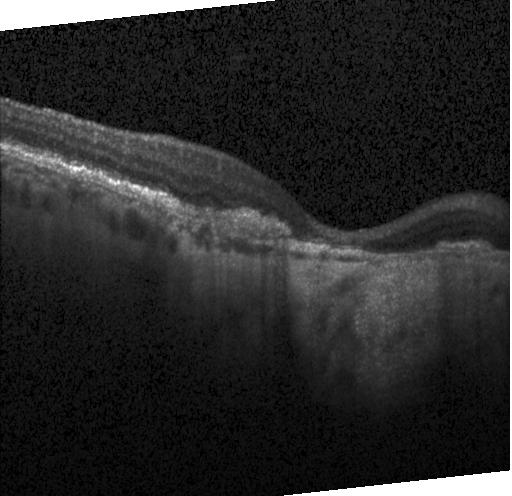 Macular scan; spectral-domain OCT; OCT B-scan; Heidelberg Spectralis.
The scan shows a choroidal neovascular membrane.